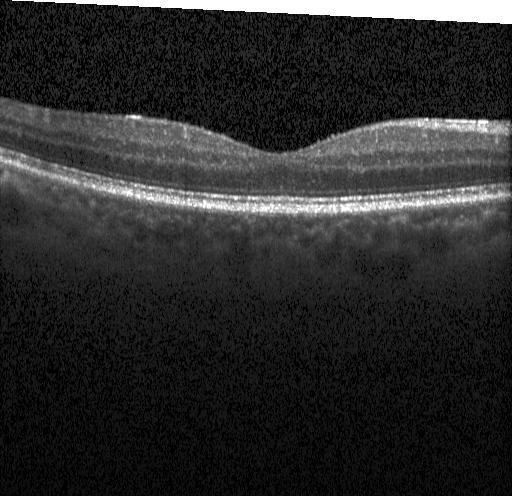

Assessment: no CNV, DME, or drusen.